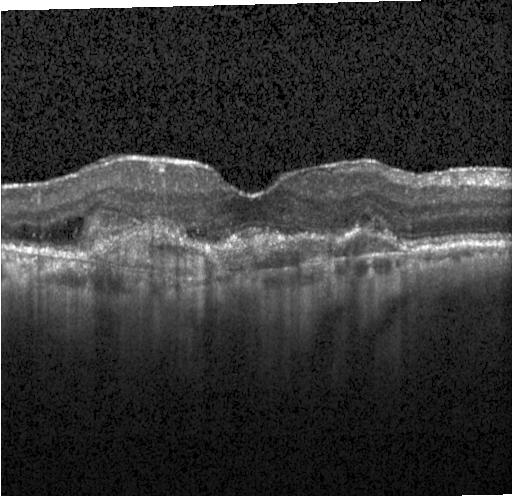

OCT B-scan showing a choroidal neovascular membrane.